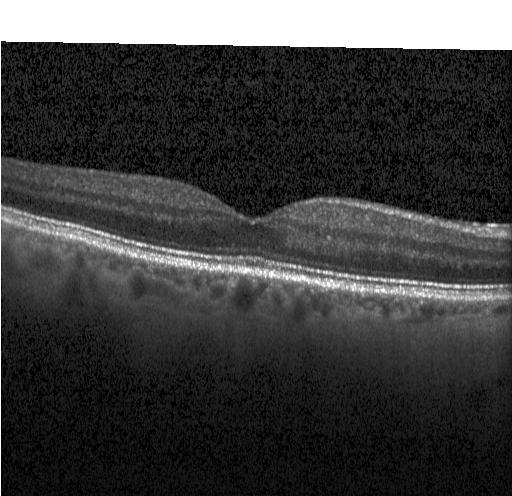 OCT finding: no CNV, no DME, and no drusen.